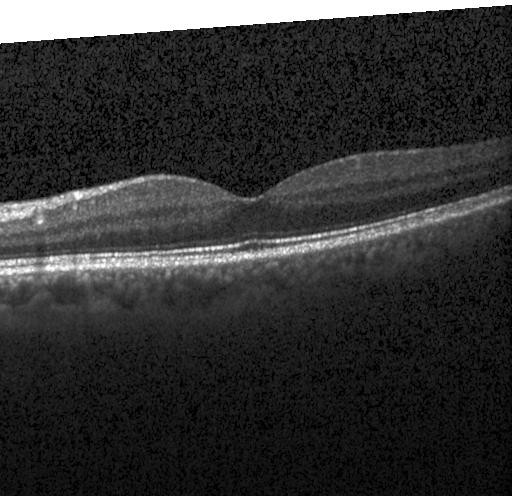

Heidelberg Spectralis; spectral-domain optical coherence tomography; retinal OCT B-scan; horizontal scan through the fovea
The scan shows no evidence of choroidal neovascularization, diabetic macular edema, or drusen.